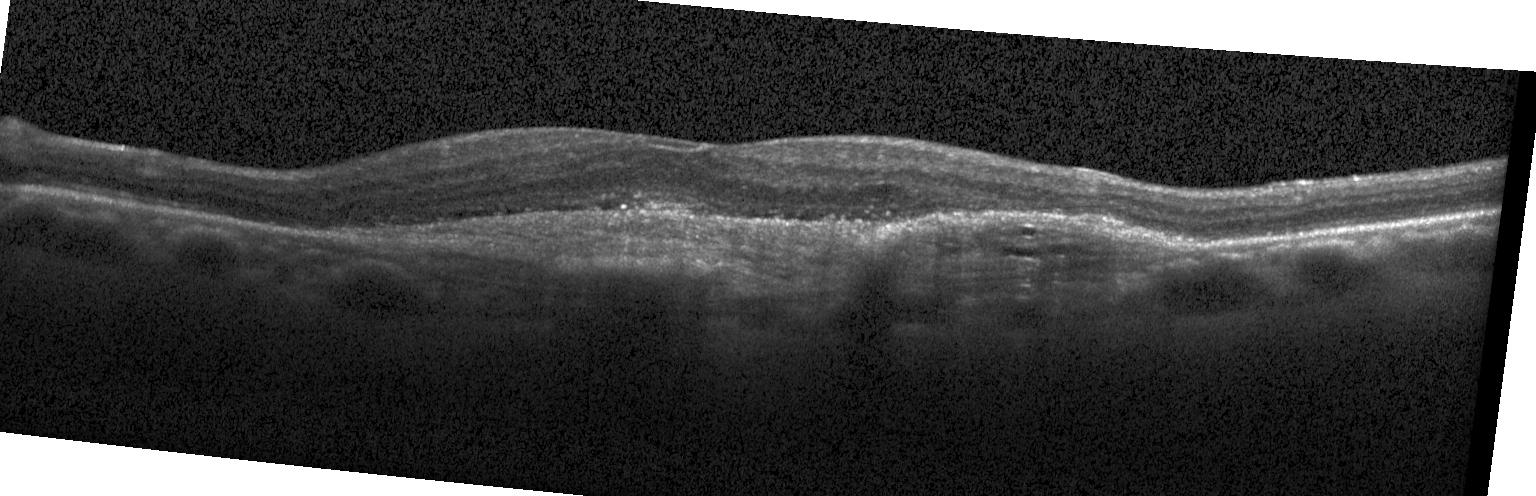

Retinal OCT cross-section
Diagnosis: choroidal neovascularization.